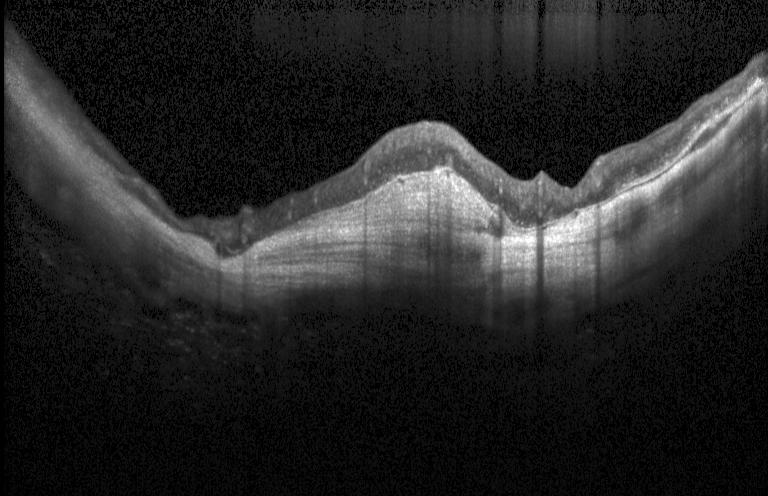

OCT finding: CNV.